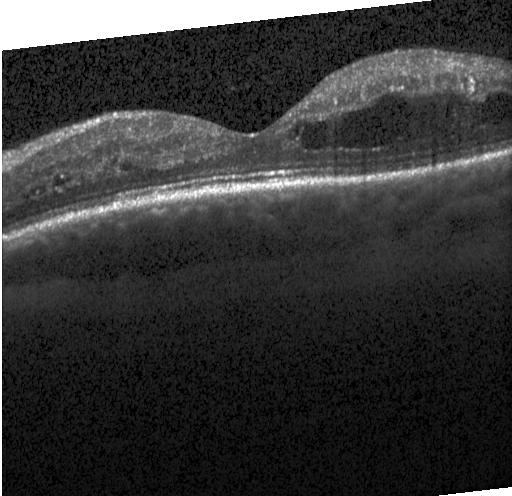
Optical coherence tomography scan, spectral-domain optical coherence tomography. The scan shows DME.